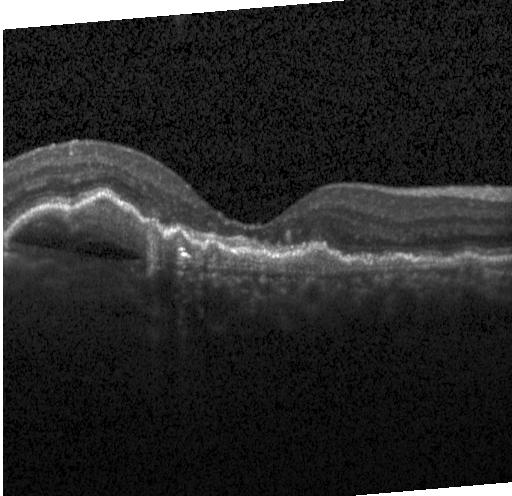 OCT line scan
This B-scan demonstrates choroidal neovascularization (CNV).